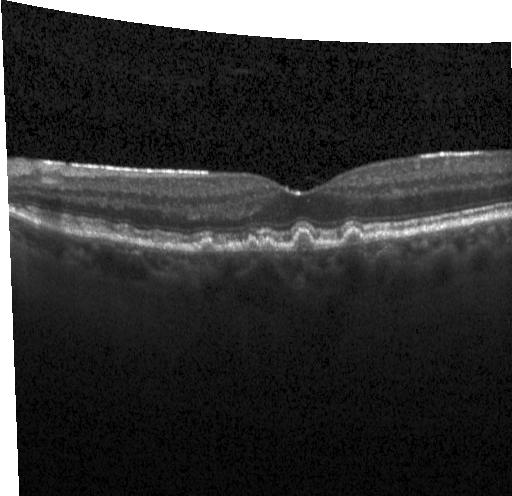
Dx: sub-RPE drusenoid deposits.